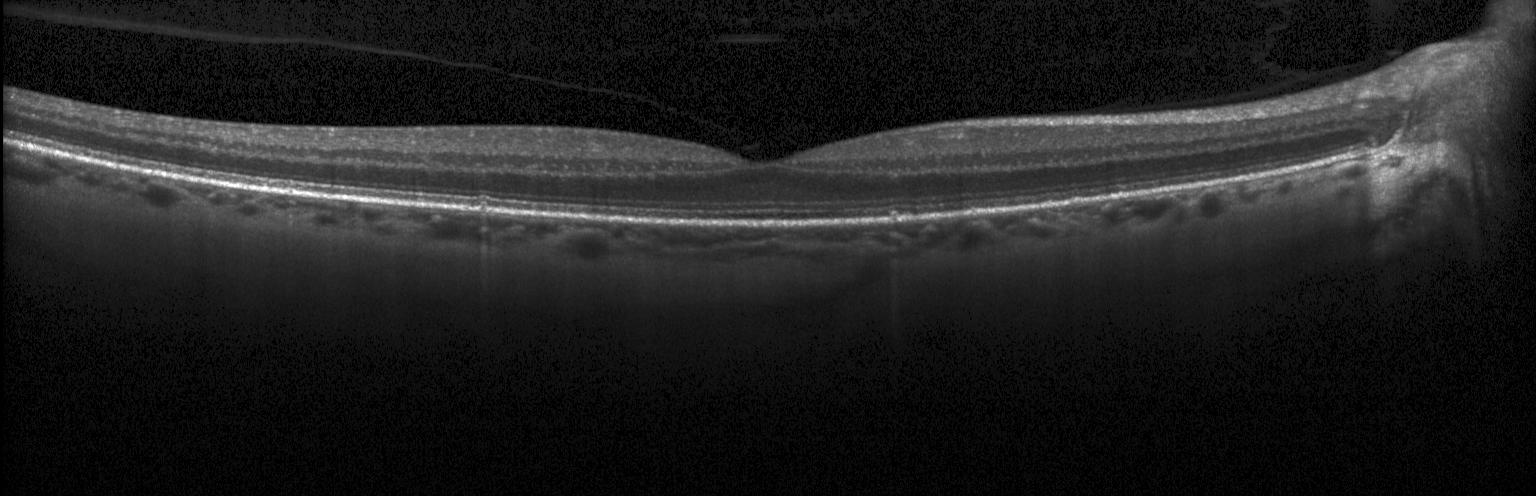

Acquired on a Heidelberg Spectralis. Optical coherence tomography B-scan. Horizontal scan through the fovea. Spectral-domain optical coherence tomography
Macular OCT: neither CNV, DME, nor drusen.